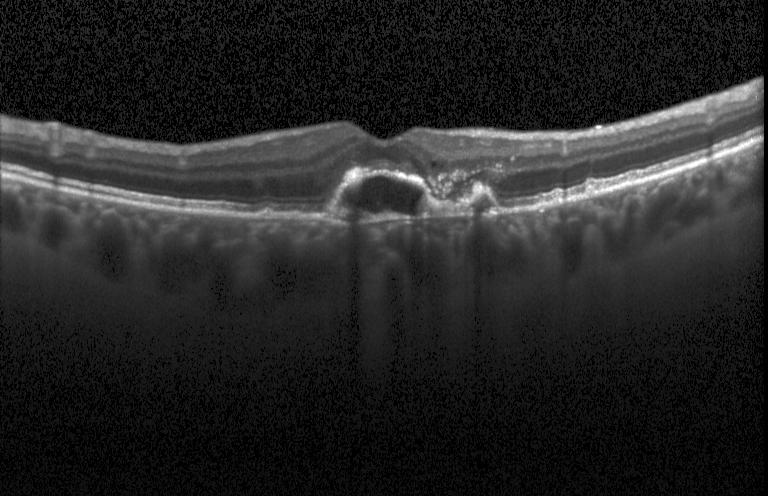
Finding: a choroidal neovascular membrane.